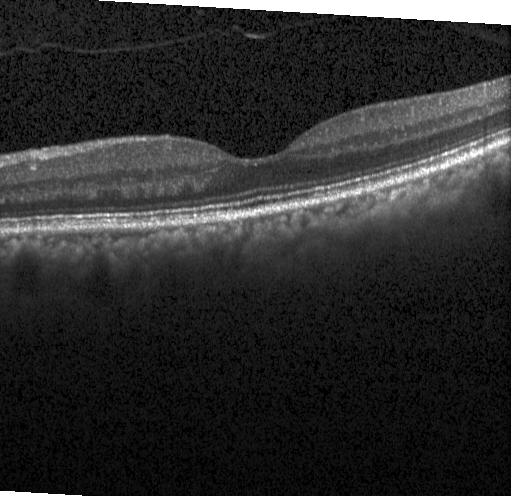

OCT line scan; acquired on a Heidelberg Spectralis; through the macula; spectral-domain optical coherence tomography — The scan shows no evidence of choroidal neovascularization, diabetic macular edema, or drusen.